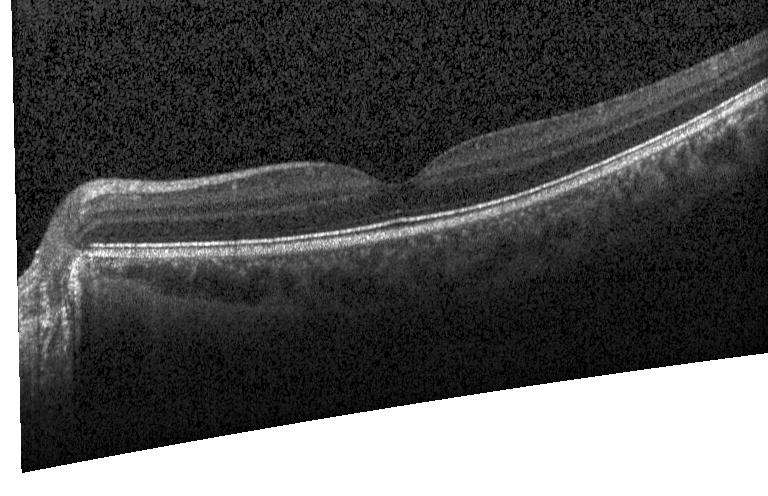

Acquired on a Heidelberg Spectralis; SD-OCT; optical coherence tomography B-scan — Finding: neither CNV, DME, nor drusen.